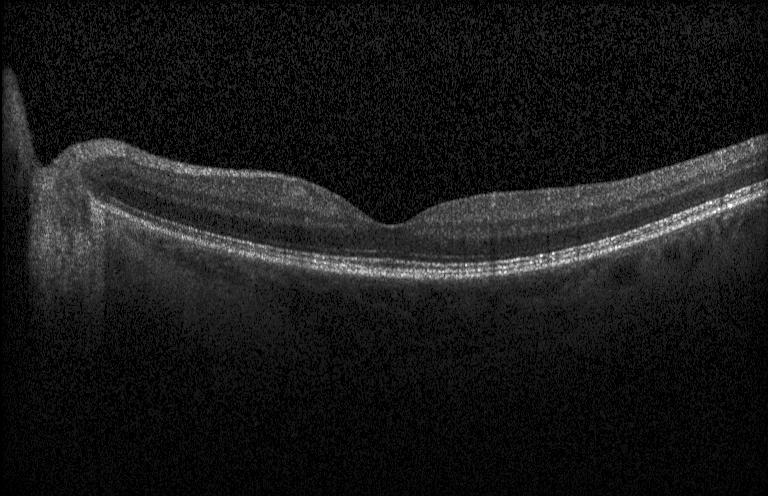 Optical coherence tomography B-scan, SD-OCT, acquired on a Heidelberg Spectralis.
The scan shows no choroidal neovascularization, diabetic macular edema, or drusen.